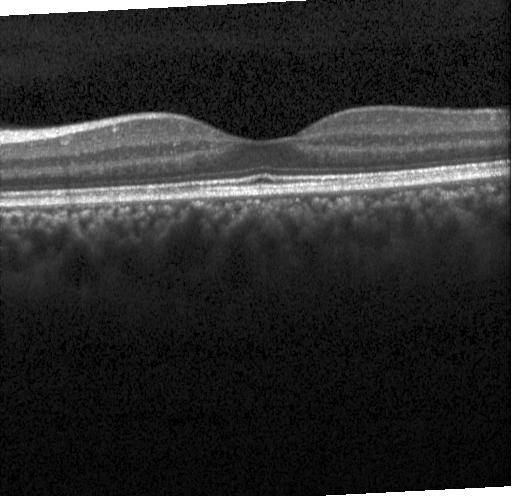
Assessment: no evidence of CNV, DME, or drusen.